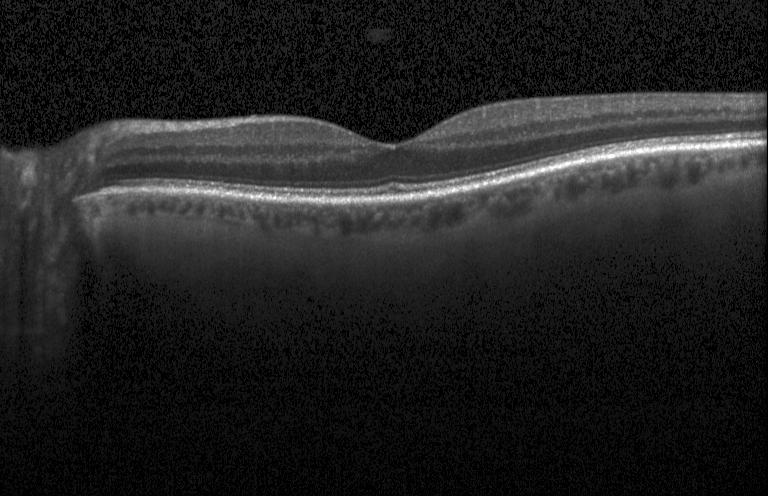

Finding: no CNV, no DME, and no drusen.